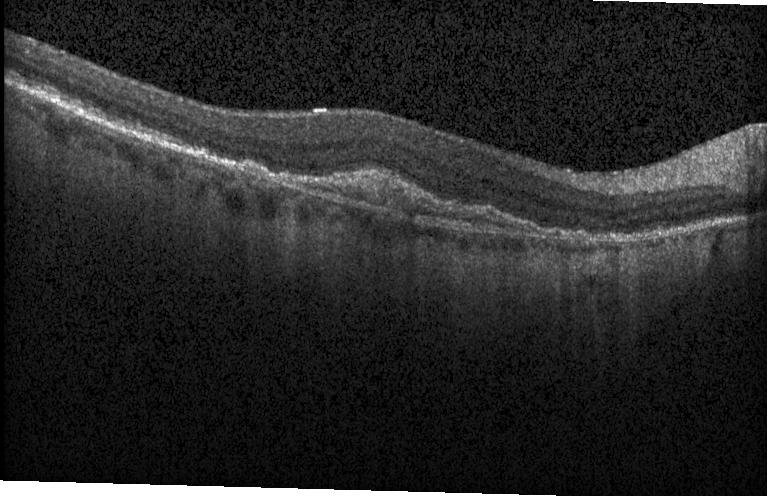 Optical coherence tomography B-scan; spectral-domain OCT; fovea-centered; acquired on a Heidelberg Spectralis — Macular OCT: CNV.